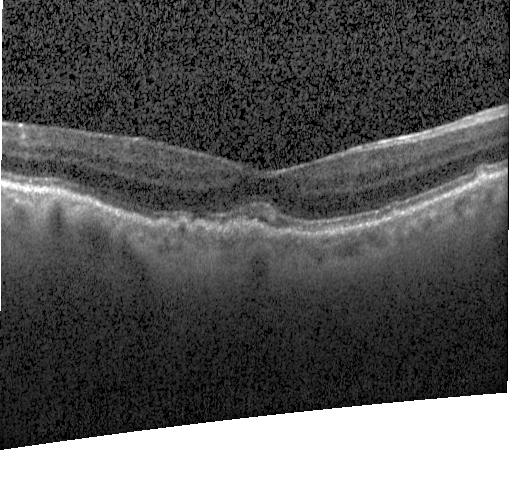

Spectral-domain OCT · fovea-centered · retinal OCT cross-section · Heidelberg Spectralis OCT system. This B-scan demonstrates choroidal neovascularization (CNV).